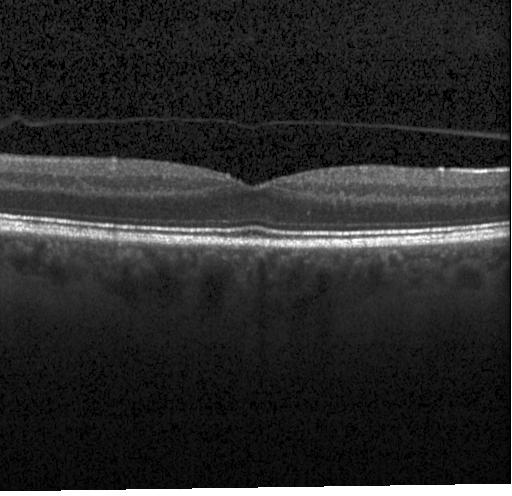

Diagnosis: no evidence of choroidal neovascularization, diabetic macular edema, or drusen.